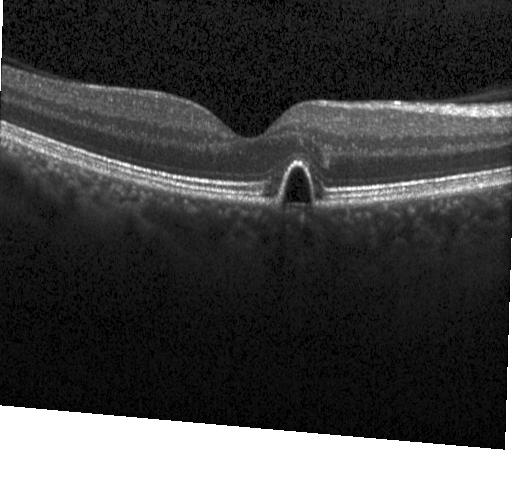 Optical coherence tomography scan · Heidelberg Spectralis · spectral-domain OCT · macular scan.
Finding: choroidal neovascularization (CNV).